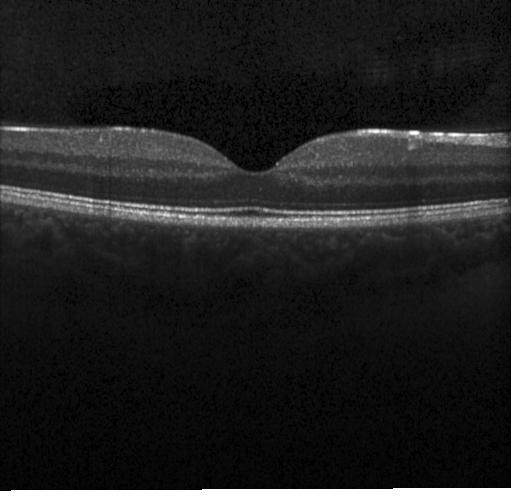 Optical coherence tomography scan. This B-scan demonstrates neither CNV, DME, nor drusen.